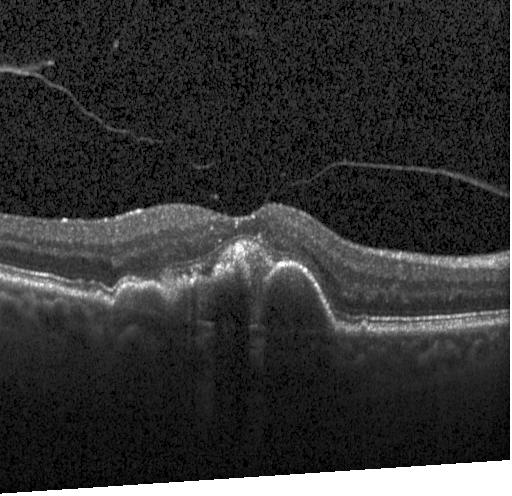
Heidelberg Spectralis OCT system. OCT line scan. Horizontal scan through the fovea. Spectral-domain OCT. Impression: a choroidal neovascular membrane.